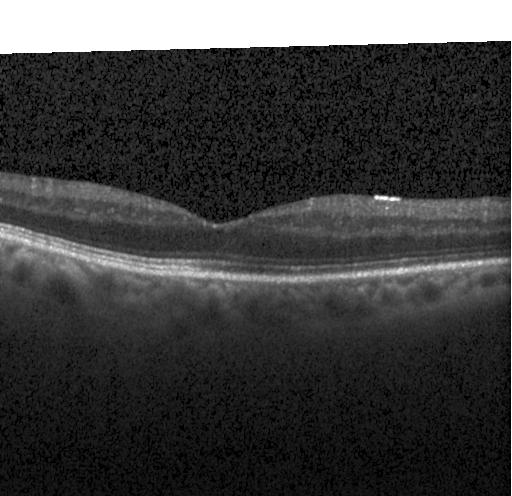 Retinal OCT cross-section showing no evidence of CNV, DME, or drusen.